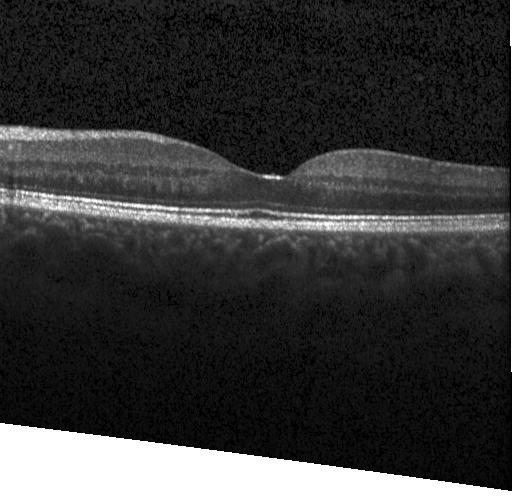

Macular OCT: no choroidal neovascularization, no diabetic macular edema, and no drusen.